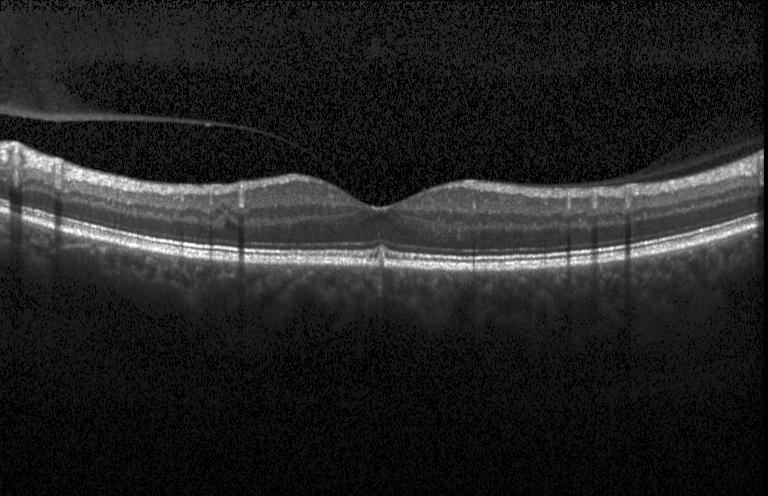

OCT scan showing sub-RPE drusenoid deposits.